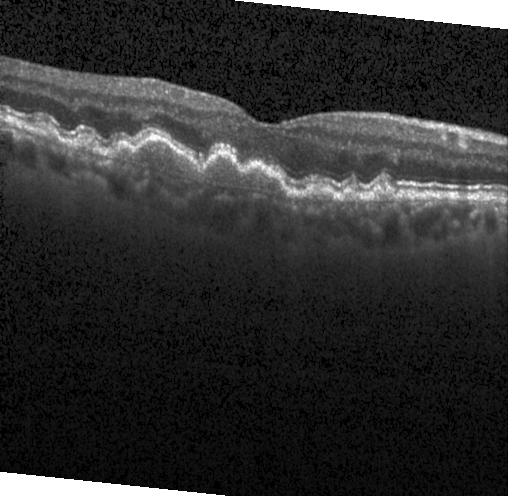

OCT B-scan. Impression: multiple drusen.